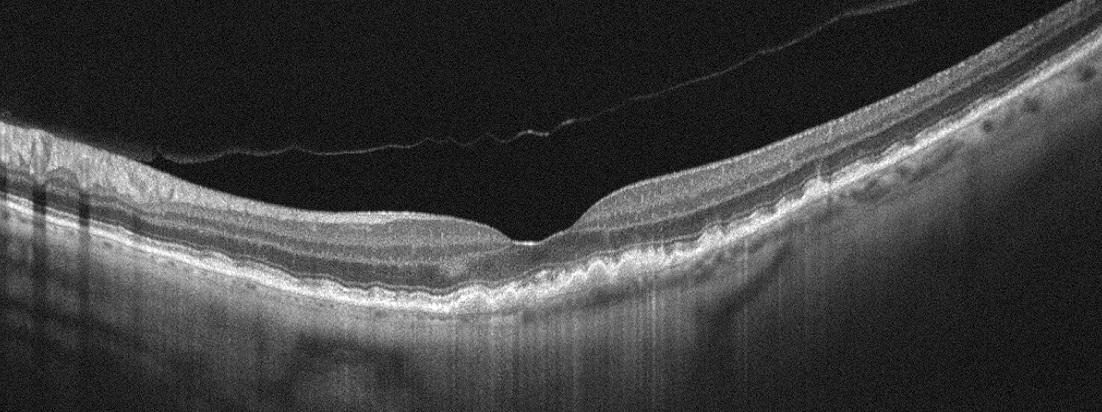
Instrument: Optovue Avanti RTVue XR · optical coherence tomography scan · fovea-centered
Dx: AMD.